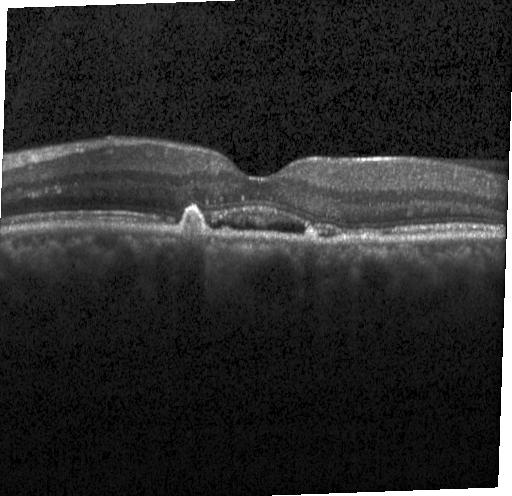
Dx: CNV.